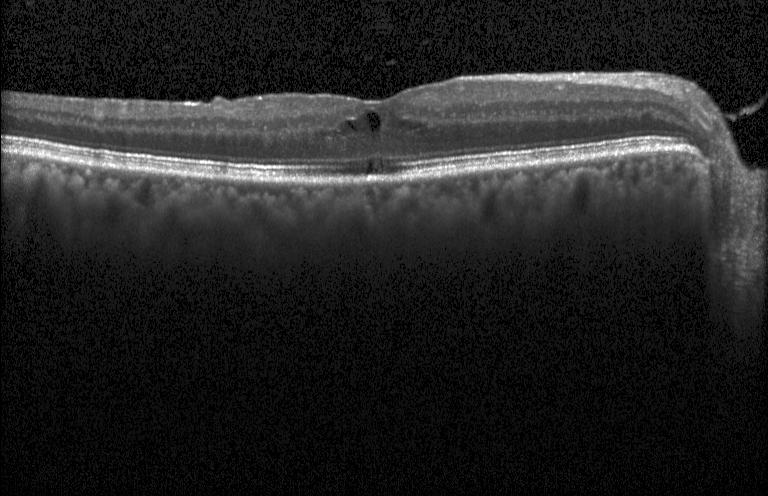
Instrument: Heidelberg Spectralis · fovea-centered · OCT line scan · spectral-domain optical coherence tomography
Macular OCT: diabetic macular edema (DME).